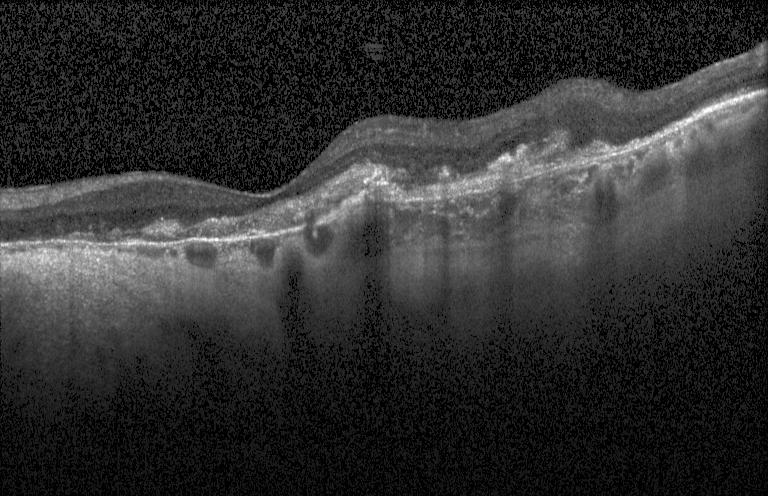
OCT B-scan, through the macula, spectral-domain OCT
Impression: a choroidal neovascular membrane.